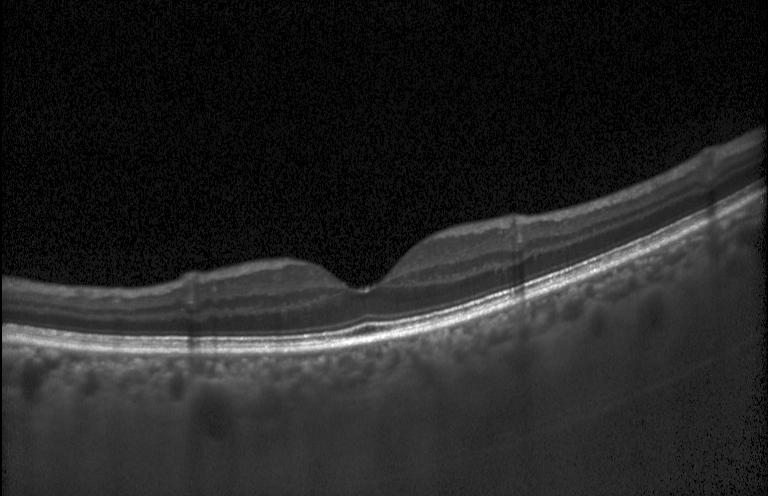
Assessment: no choroidal neovascularization, no diabetic macular edema, and no drusen.